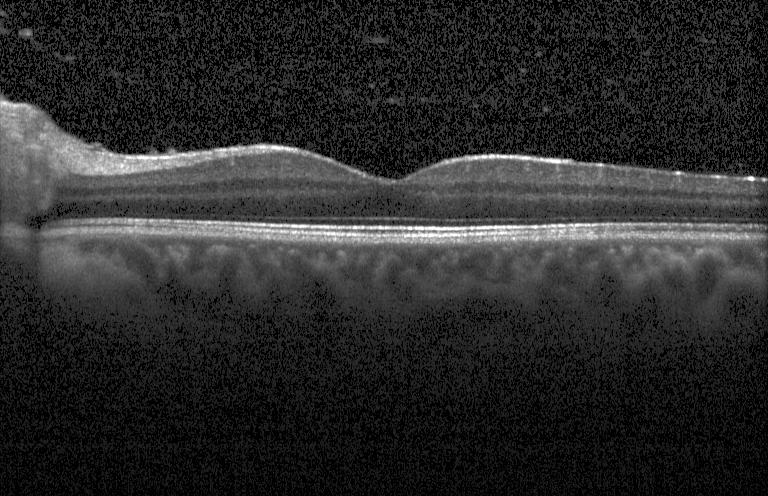

Retinal OCT B-scan — Diagnosis: no evidence of choroidal neovascularization, diabetic macular edema, or drusen.